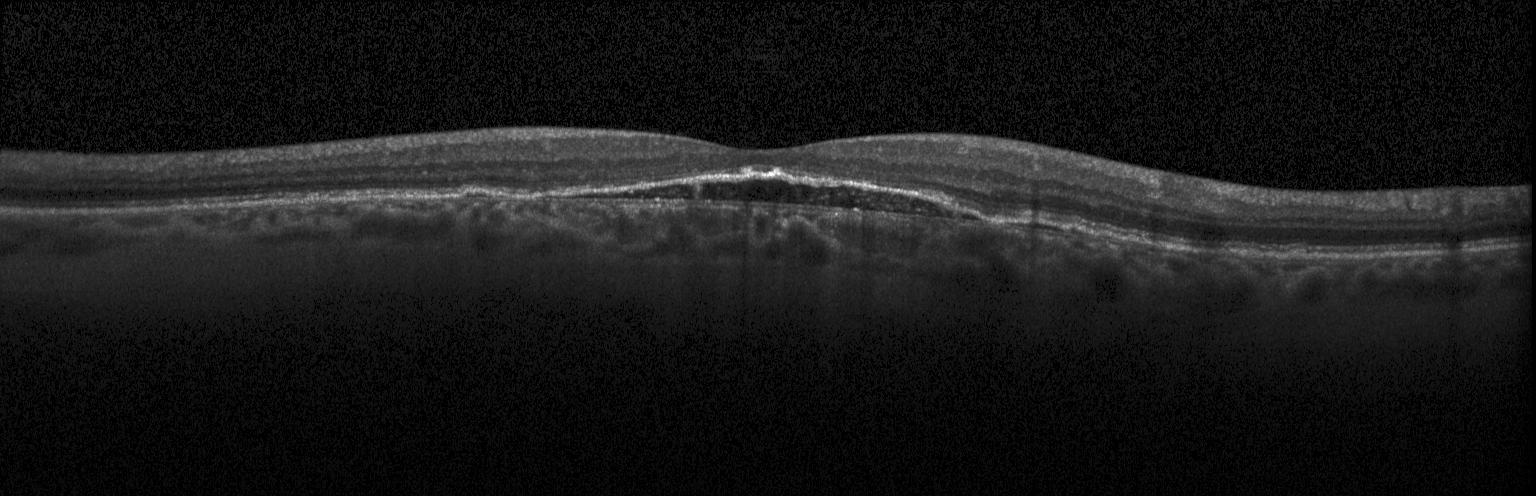 Through the macula, OCT B-scan, Heidelberg Spectralis OCT system.
Finding: a choroidal neovascular membrane.